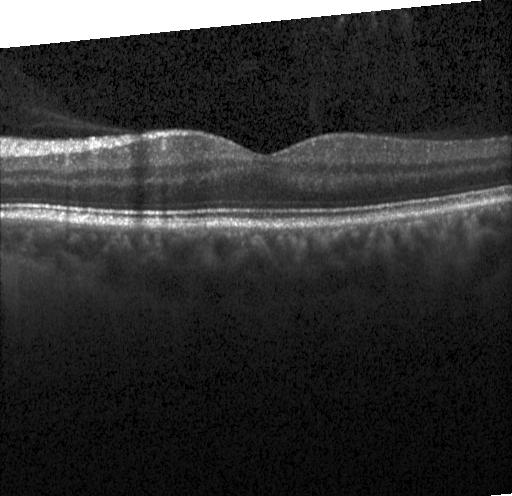 SD-OCT · instrument: Heidelberg Spectralis · OCT line scan · centered on the fovea — Assessment: neither choroidal neovascularization, diabetic macular edema, nor drusen.